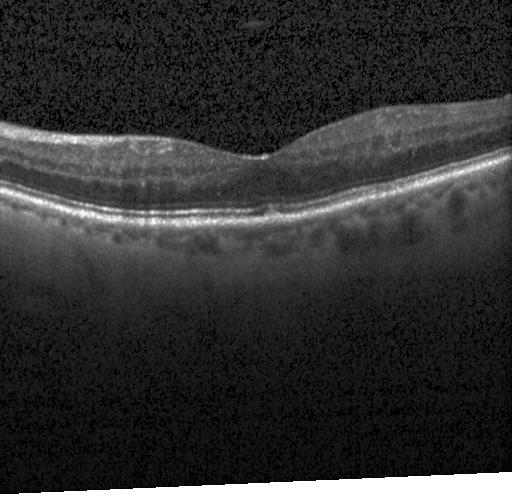
Diagnosis: multiple drusen.